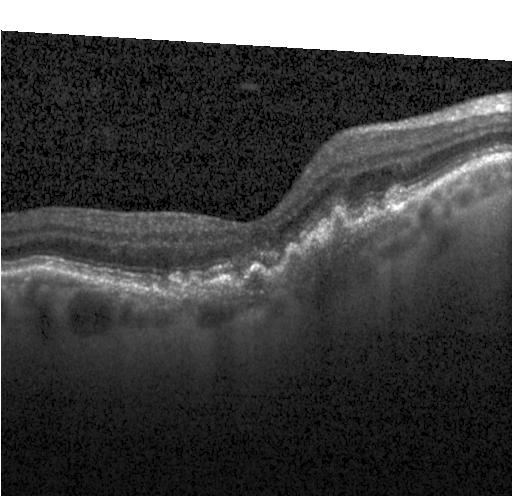

Retinal OCT cross-section. Macular scan. Macular OCT: CNV.